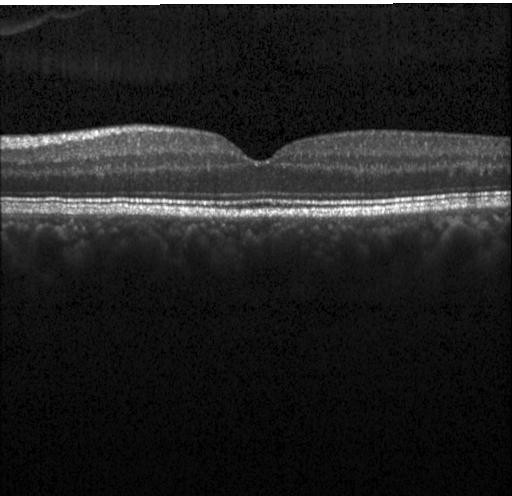
Retinal OCT B-scan; Heidelberg Spectralis OCT system.
OCT finding: no choroidal neovascularization, no diabetic macular edema, and no drusen.